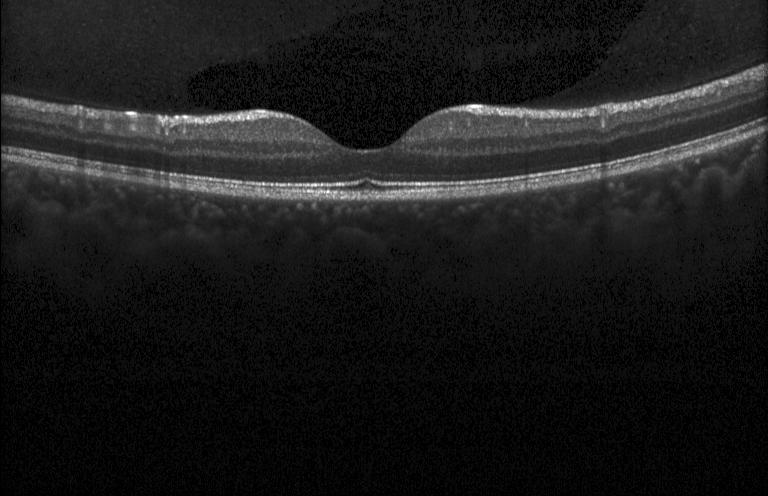
OCT line scan. Spectral-domain OCT. Fovea-centered. Acquired on a Heidelberg Spectralis
No evidence of CNV, DME, or drusen.